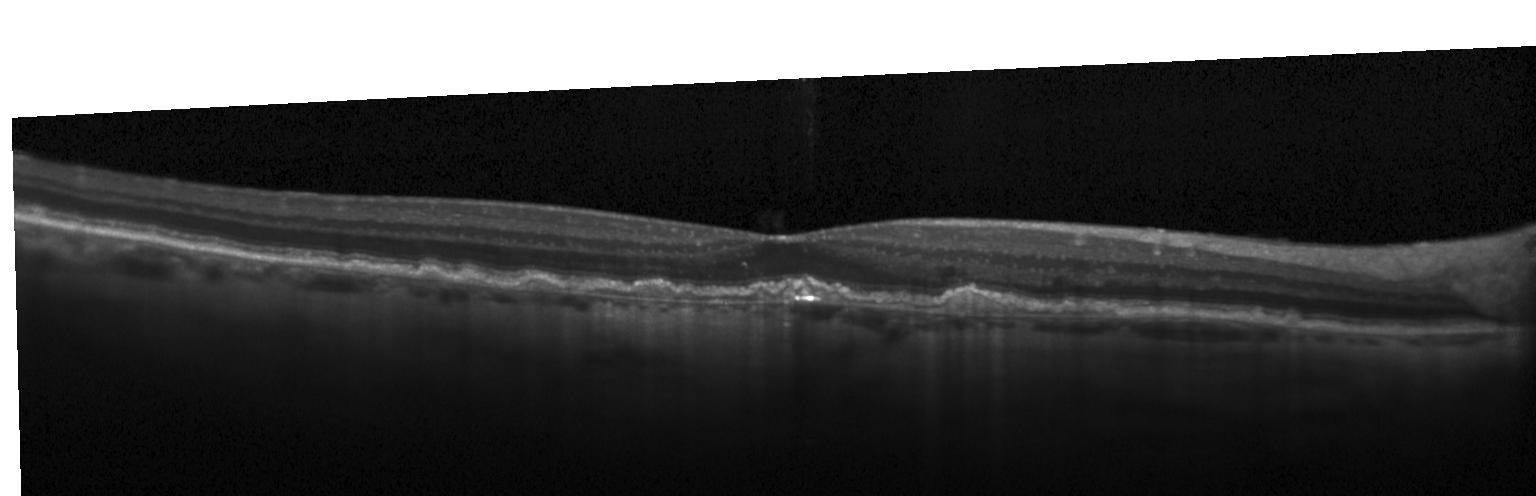
Acquired on a Heidelberg Spectralis · retinal OCT cross-section · spectral-domain OCT.
Assessment: CNV.